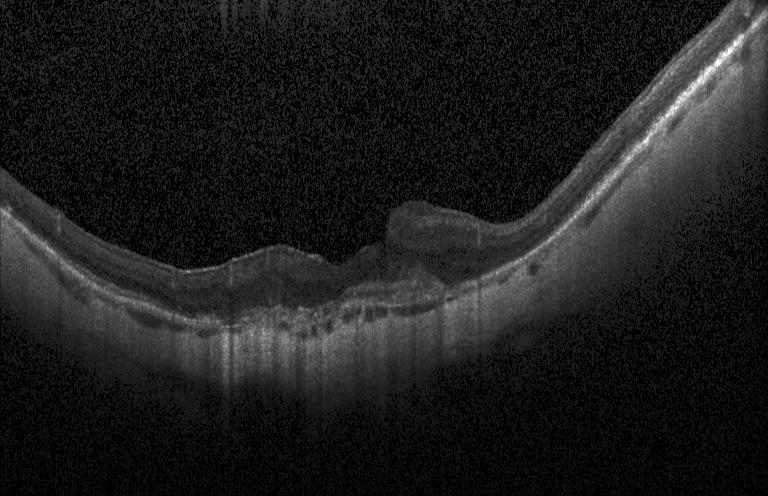
Retinal OCT cross-section.
This B-scan demonstrates CNV.